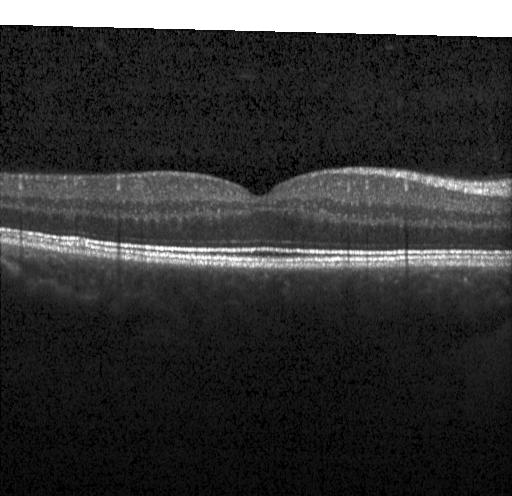

OCT line scan — Macular OCT: no choroidal neovascularization, diabetic macular edema, or drusen.